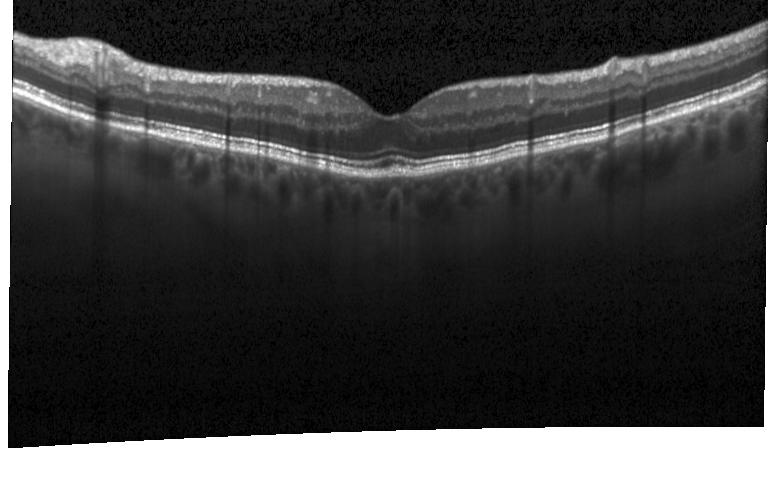
Through the macula. OCT B-scan. Spectral-domain optical coherence tomography — Assessment: neither choroidal neovascularization, diabetic macular edema, nor drusen.